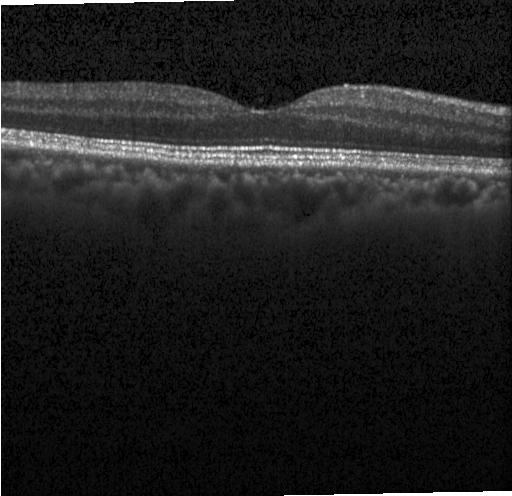 Dx: no choroidal neovascularization, no diabetic macular edema, and no drusen.